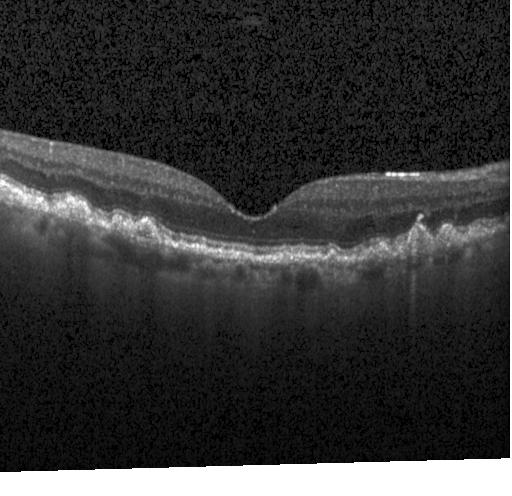

Macular OCT demonstrating multiple drusen.